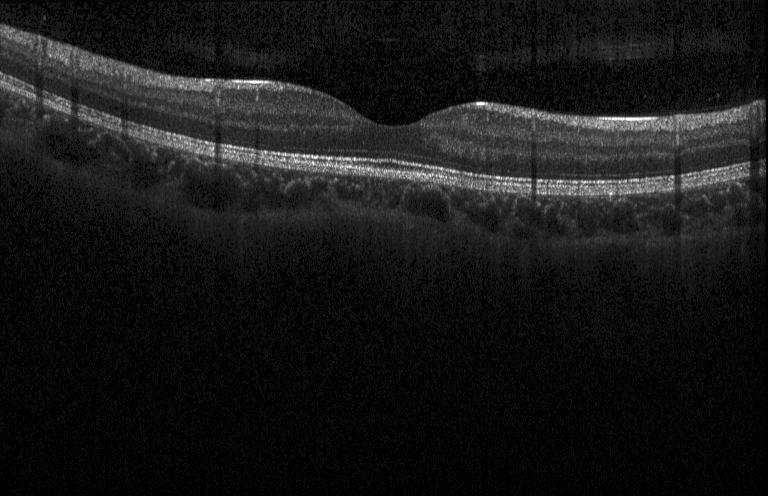
Finding: no CNV, no DME, and no drusen.